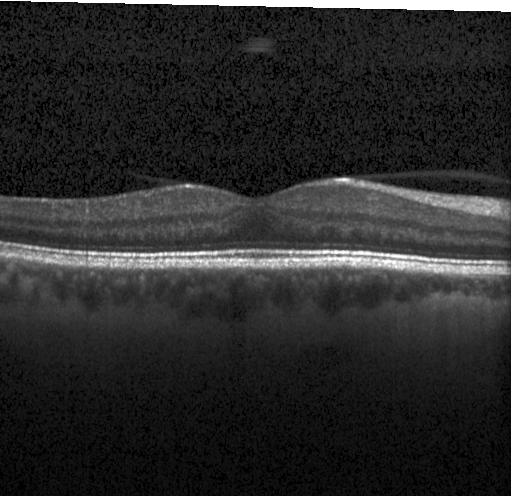

OCT finding: no CNV, DME, or drusen.